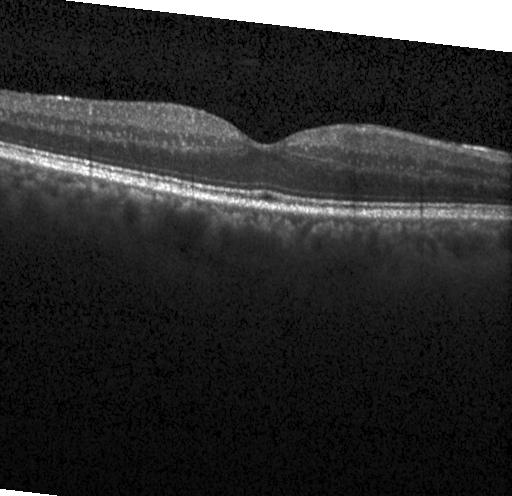
Spectral-domain OCT B-scan: no choroidal neovascularization, no diabetic macular edema, and no drusen.